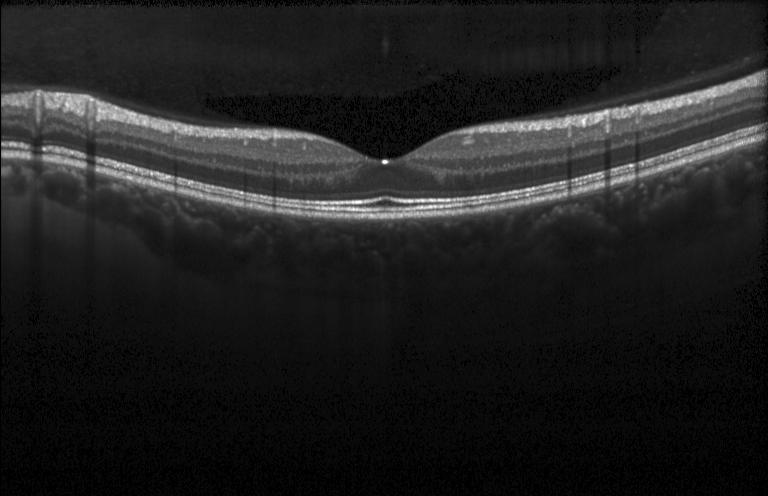
Retinal OCT cross-section showing no evidence of CNV, DME, or drusen.